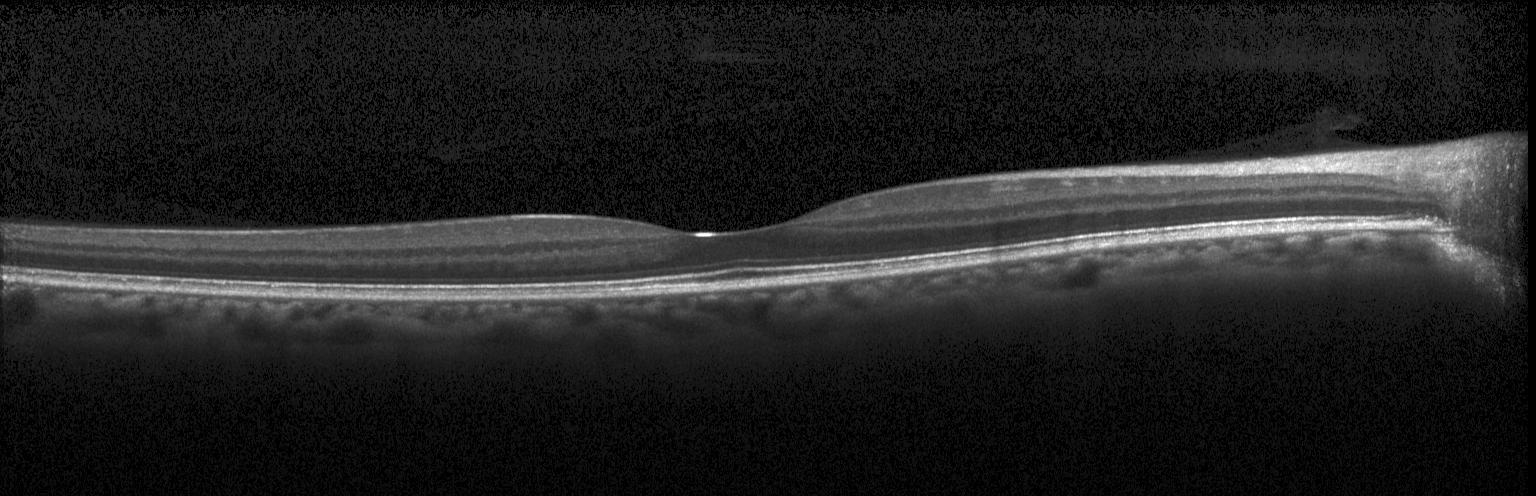
Diagnosis: neither choroidal neovascularization, diabetic macular edema, nor drusen.